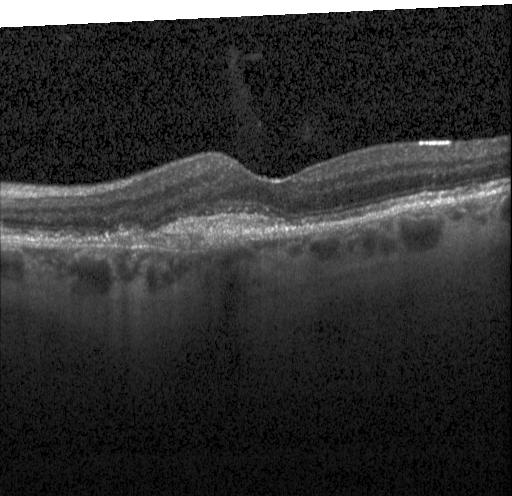

Finding: choroidal neovascularization.